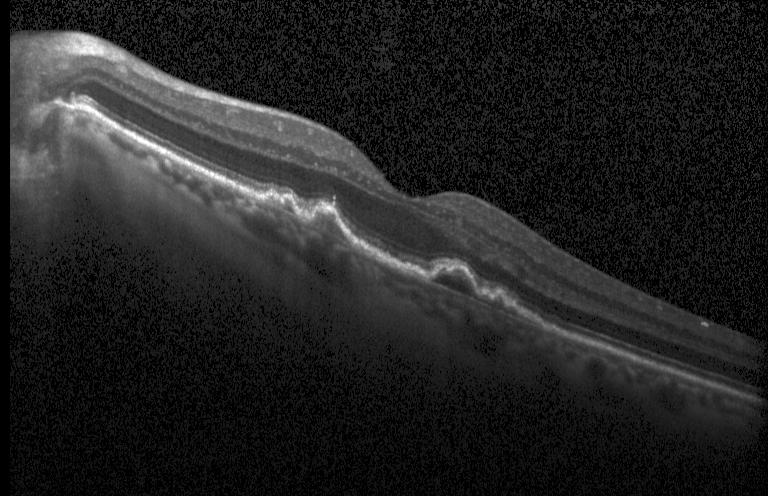
Macular OCT demonstrating drusen.